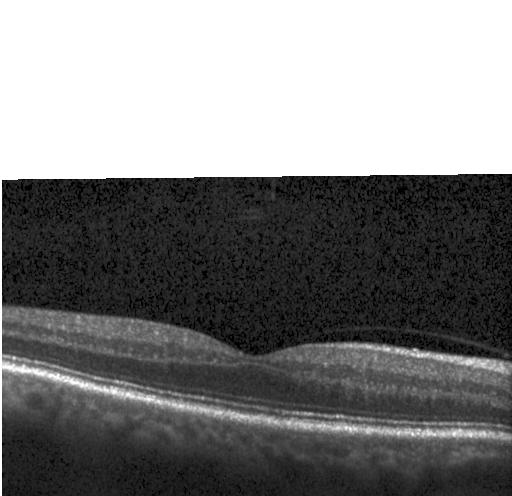 Retinal OCT cross-section. Acquired on a Heidelberg Spectralis. Through the macula.
Macular OCT: no choroidal neovascularization, no diabetic macular edema, and no drusen.